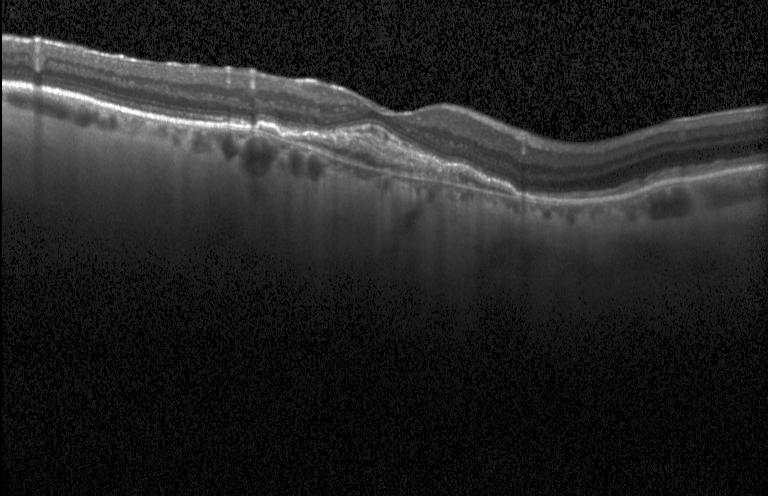
Diagnosis: a choroidal neovascular membrane.